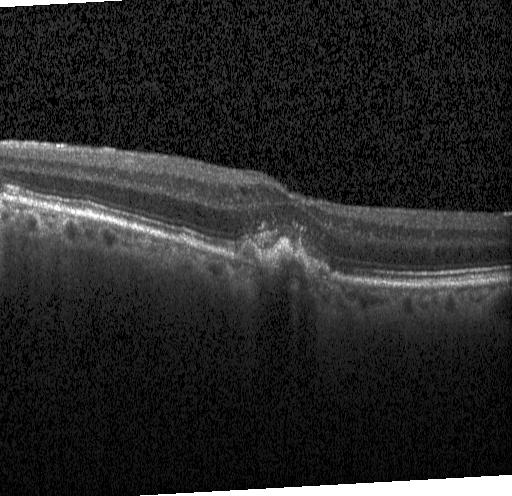
Retinal OCT cross-section showing choroidal neovascularization (CNV).